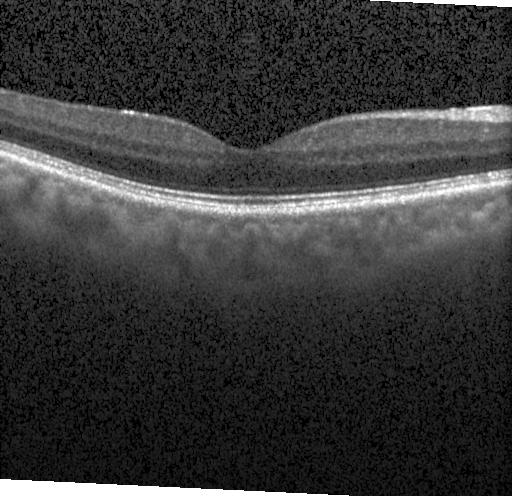 OCT line scan, spectral-domain optical coherence tomography. This B-scan demonstrates no choroidal neovascularization, no diabetic macular edema, and no drusen.